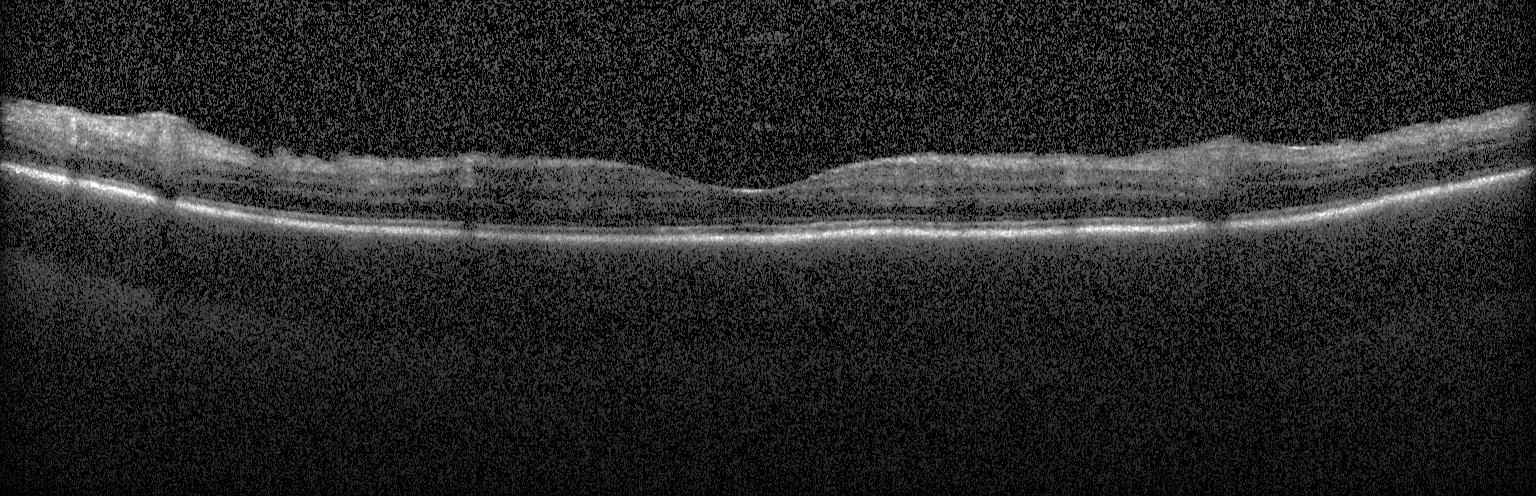

OCT line scan, spectral-domain optical coherence tomography, horizontal scan through the fovea, instrument: Heidelberg Spectralis — Assessment: no choroidal neovascularization, diabetic macular edema, or drusen.